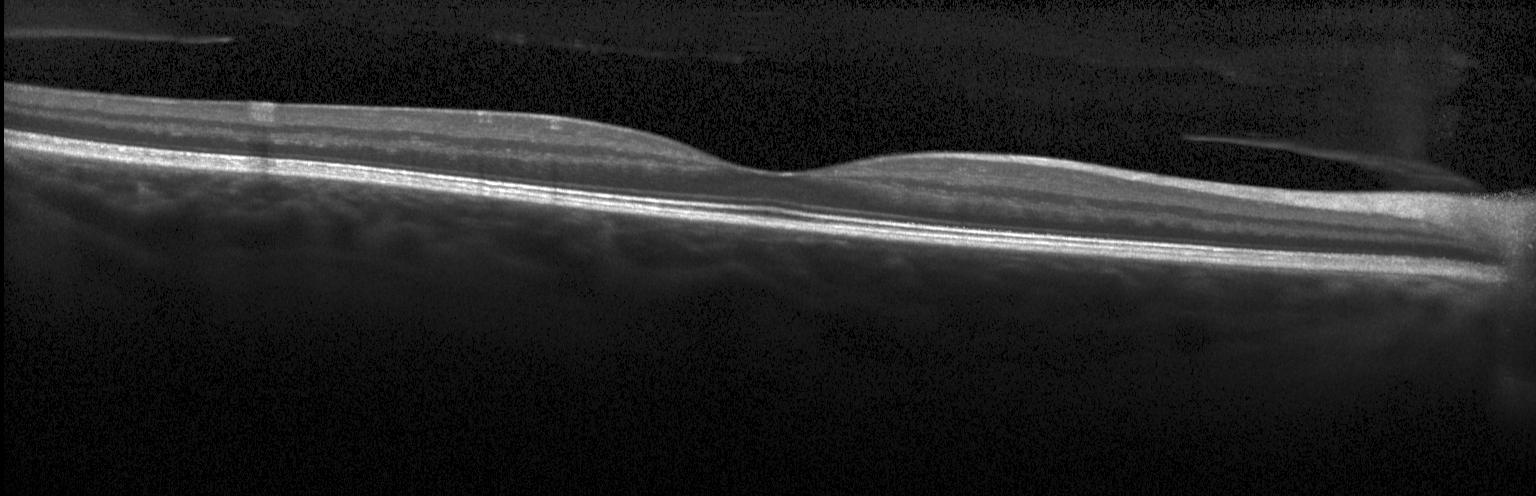
Macular scan; spectral-domain OCT; acquired on a Heidelberg Spectralis; OCT line scan
Assessment: neither CNV, DME, nor drusen.